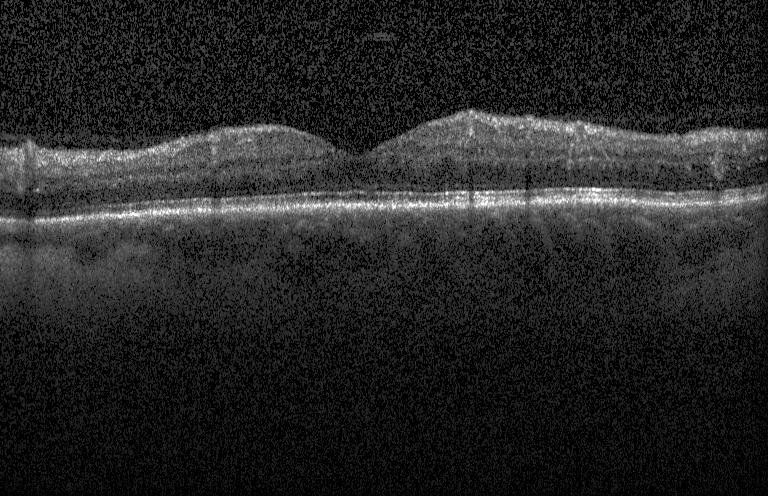

Assessment: DME.